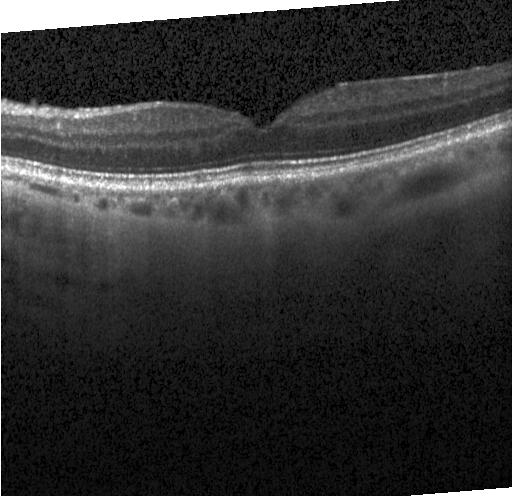
Macular OCT demonstrating no evidence of CNV, DME, or drusen.